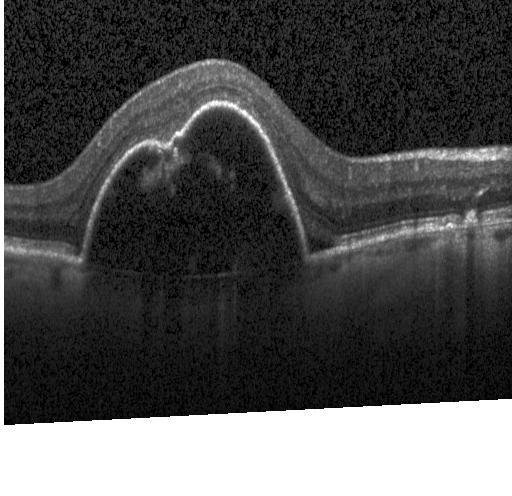 Macular scan, acquired on a Heidelberg Spectralis, OCT B-scan. Diagnosis: choroidal neovascularization.